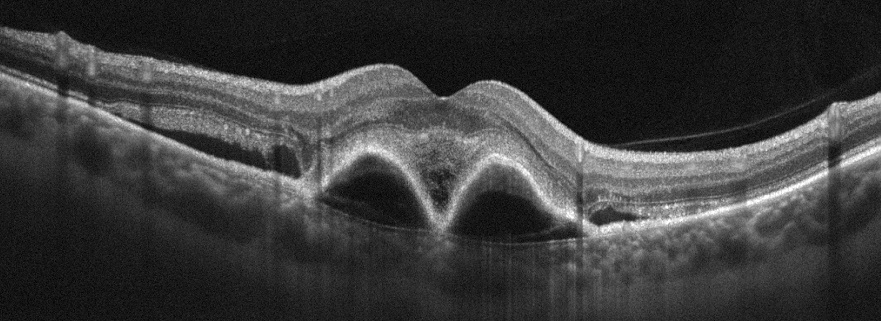 Macular scan; Optovue Avanti RTVue XR; OCT B-scan.
Assessment: AMD.